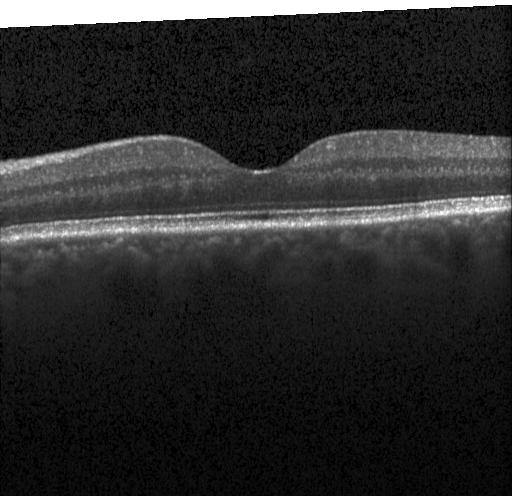 OCT B-scan.
Impression: no evidence of choroidal neovascularization, diabetic macular edema, or drusen.